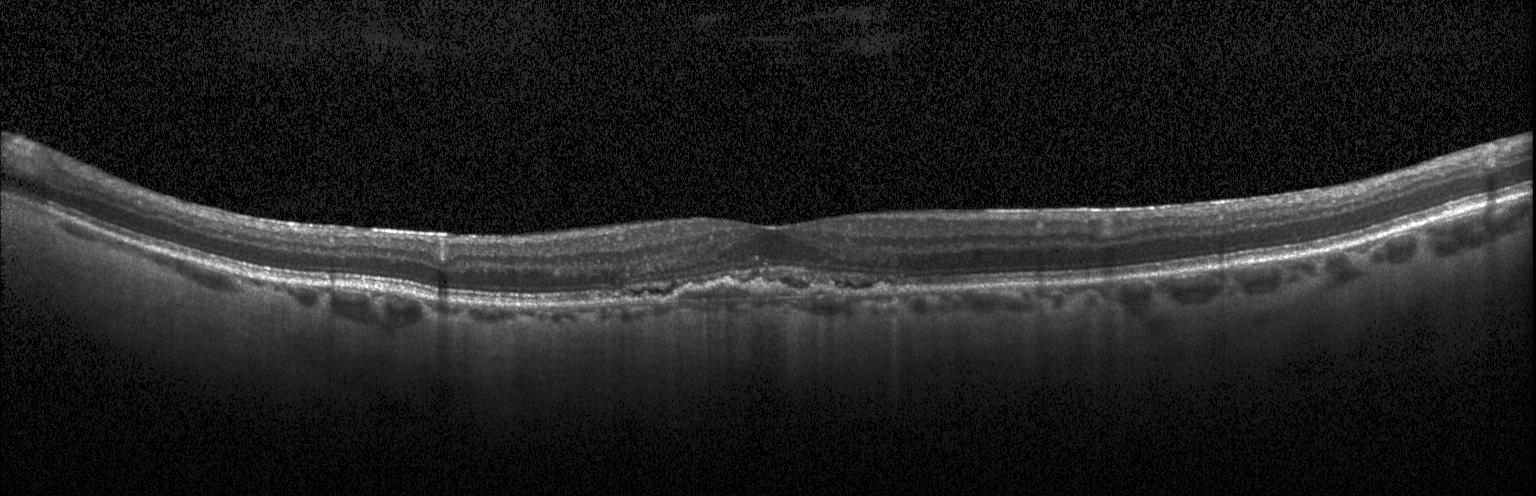
Finding: a choroidal neovascular membrane.